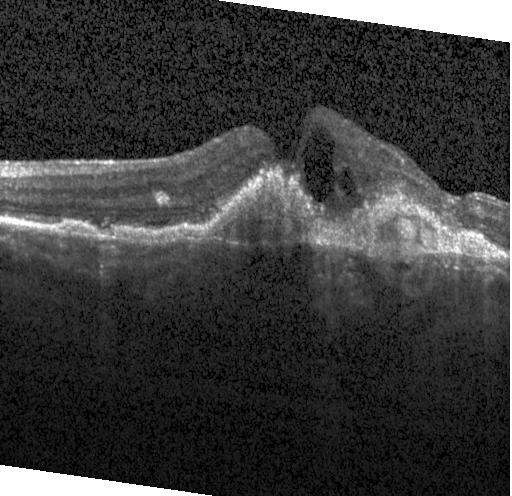

Spectral-domain OCT; through the macula; Heidelberg Spectralis; optical coherence tomography scan.
This B-scan demonstrates choroidal neovascularization.